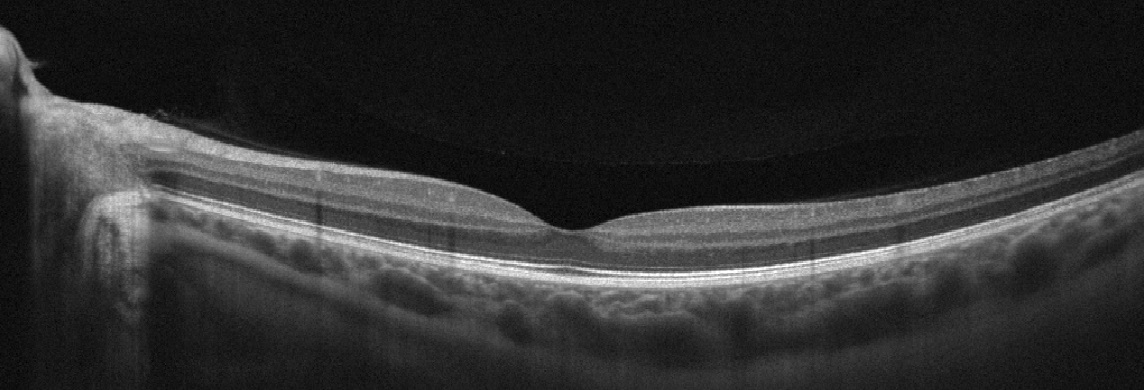

Finding: no evidence of AMD, DME, ERM, RAO, RVO, or VID.